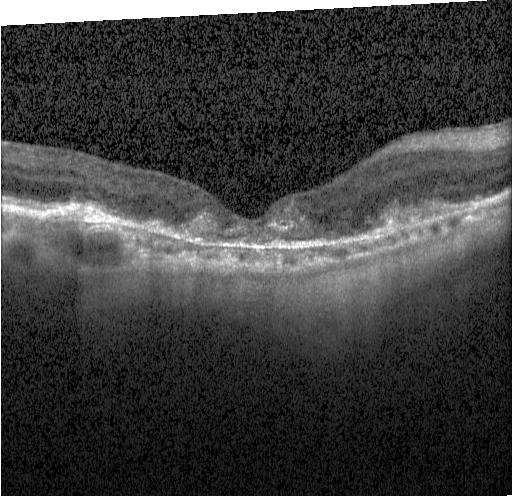 The scan shows choroidal neovascularization.